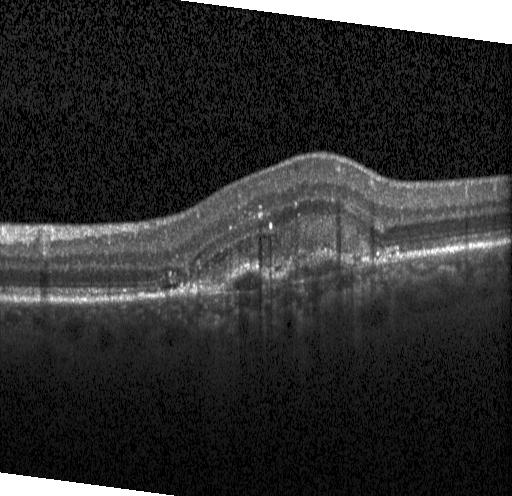 OCT B-scan showing a choroidal neovascular membrane.